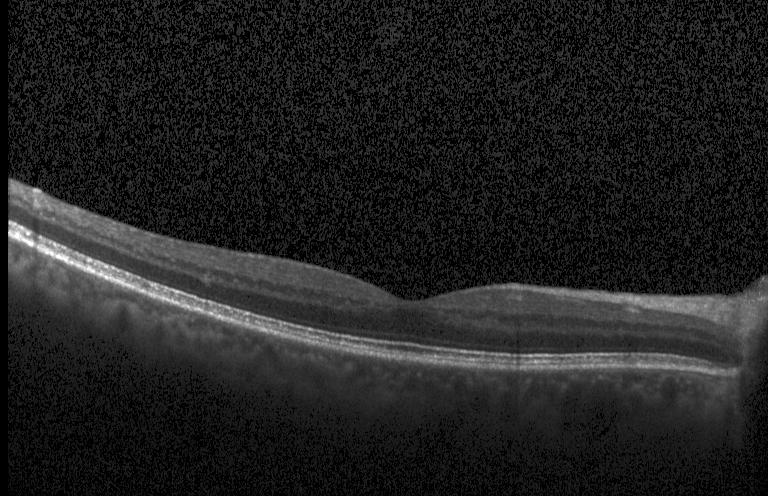

Horizontal scan through the fovea, spectral-domain OCT, retinal OCT B-scan. Diagnosis: no evidence of choroidal neovascularization, diabetic macular edema, or drusen.